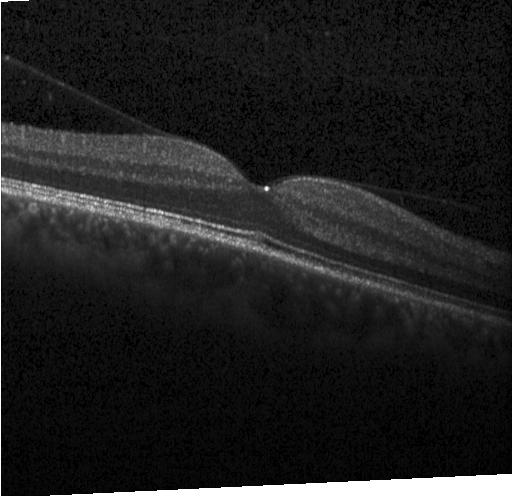
Optical coherence tomography scan
This B-scan demonstrates no CNV, DME, or drusen.